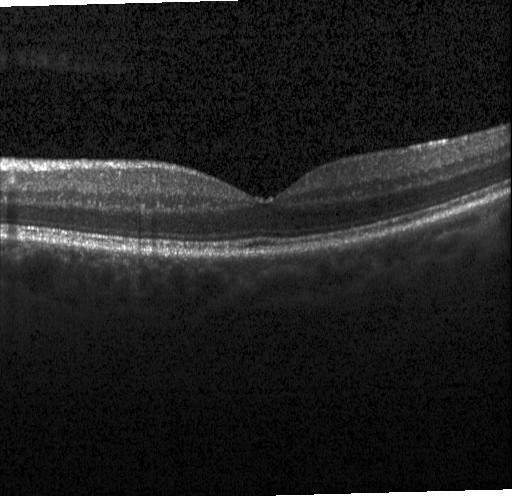

Retinal OCT cross-section. Instrument: Heidelberg Spectralis — Assessment: no evidence of choroidal neovascularization, diabetic macular edema, or drusen.